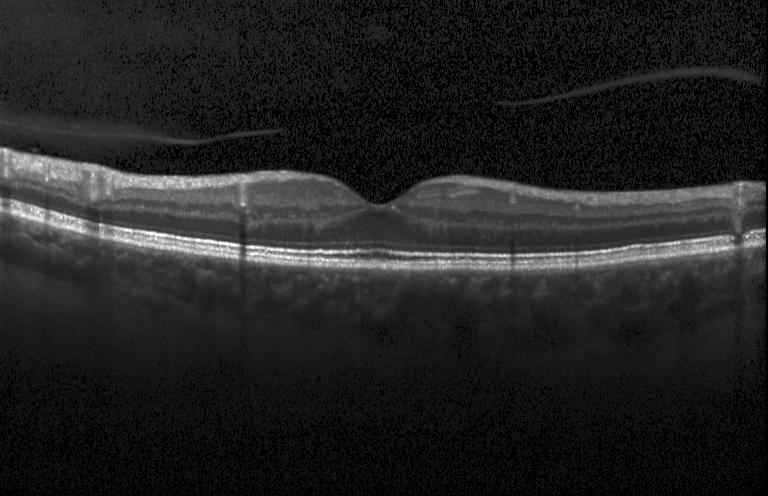
Retinal OCT cross-section. Heidelberg Spectralis OCT system
Macular OCT: no evidence of choroidal neovascularization, diabetic macular edema, or drusen.